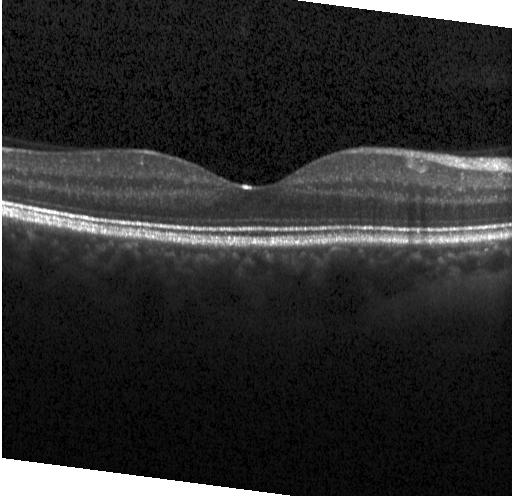
Dx: no choroidal neovascularization, diabetic macular edema, or drusen.